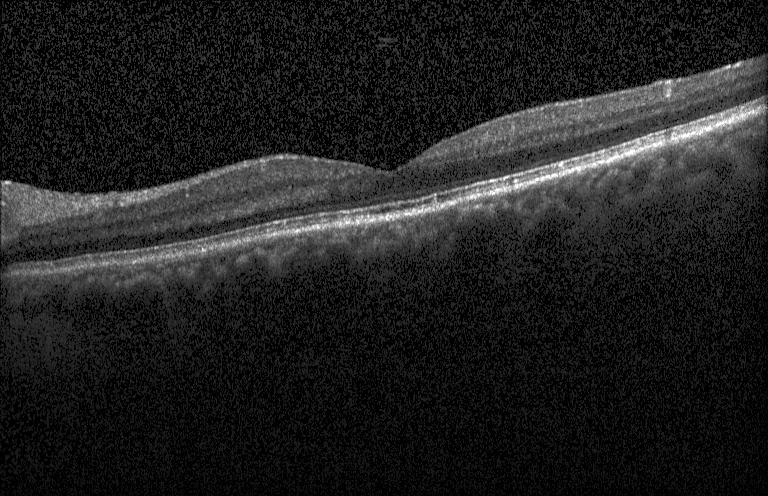

Diagnosis: no evidence of choroidal neovascularization, diabetic macular edema, or drusen.